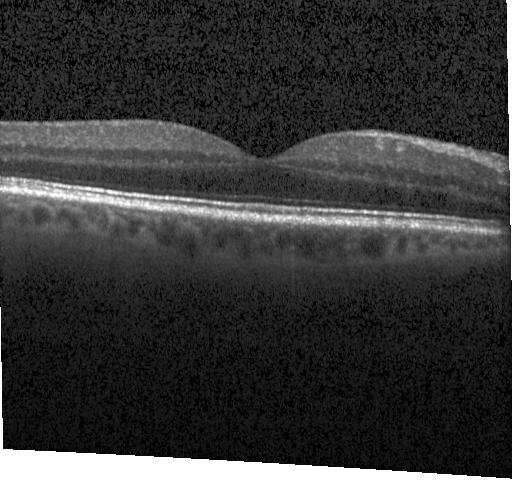 Finding: no evidence of choroidal neovascularization, diabetic macular edema, or drusen.